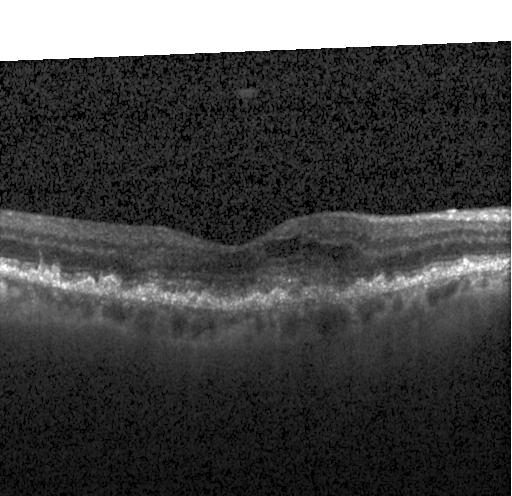

OCT finding: choroidal neovascularization (CNV).